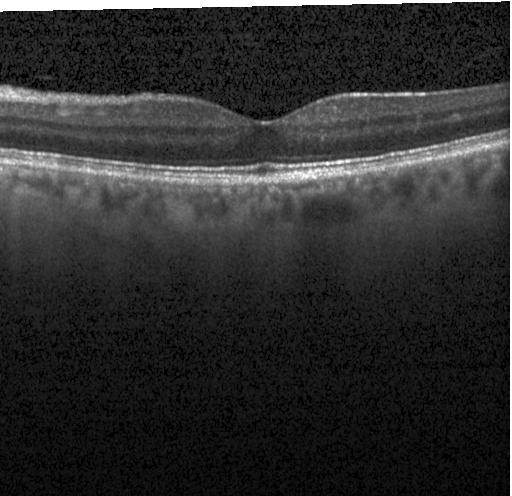
OCT line scan, instrument: Heidelberg Spectralis
Finding: no CNV, DME, or drusen.